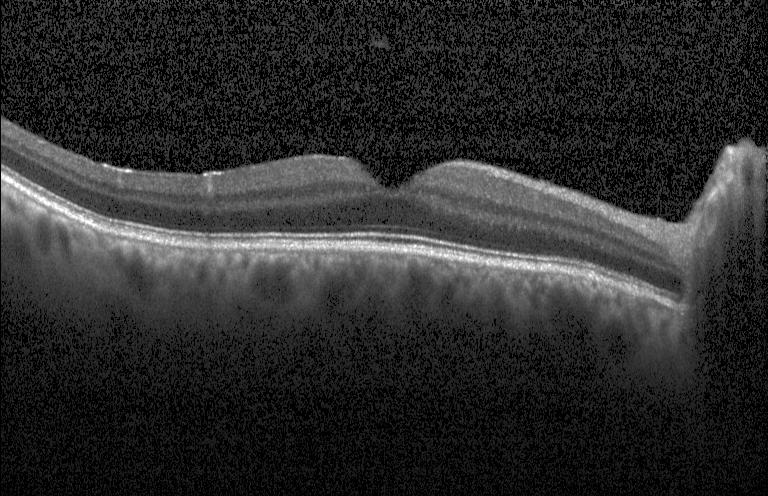
Heidelberg Spectralis OCT system; spectral-domain OCT; OCT B-scan
OCT finding: neither choroidal neovascularization, diabetic macular edema, nor drusen.